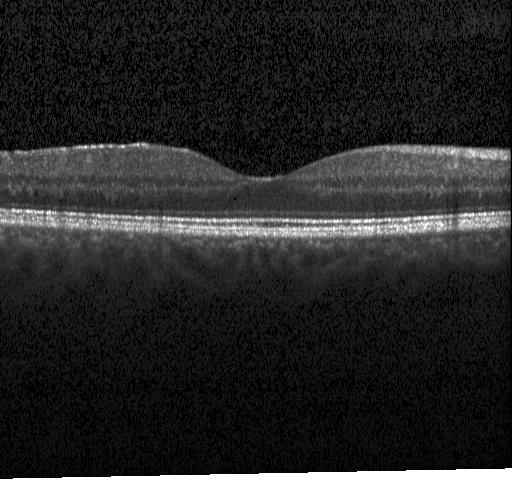 OCT line scan. The scan shows no choroidal neovascularization, diabetic macular edema, or drusen.